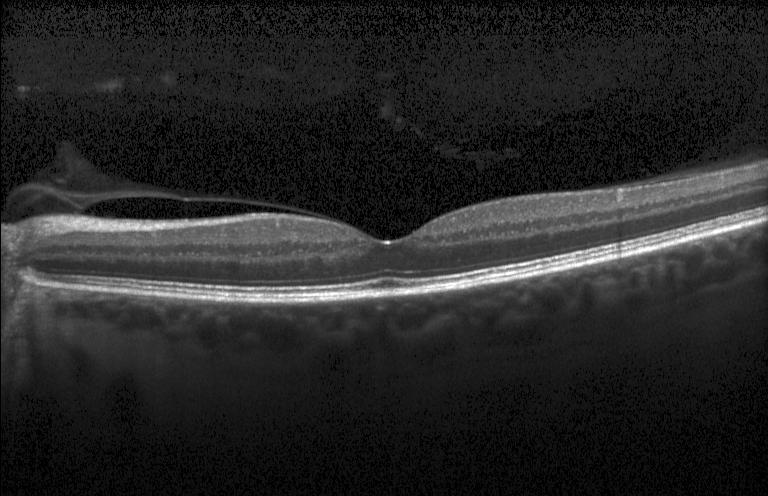

OCT line scan — The scan shows no CNV, no DME, and no drusen.